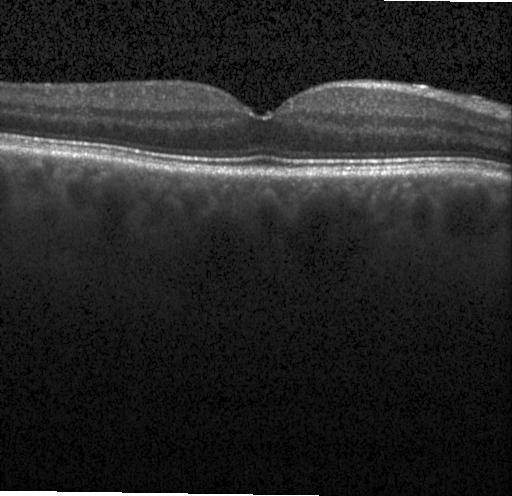 Diagnosis: no CNV, DME, or drusen.